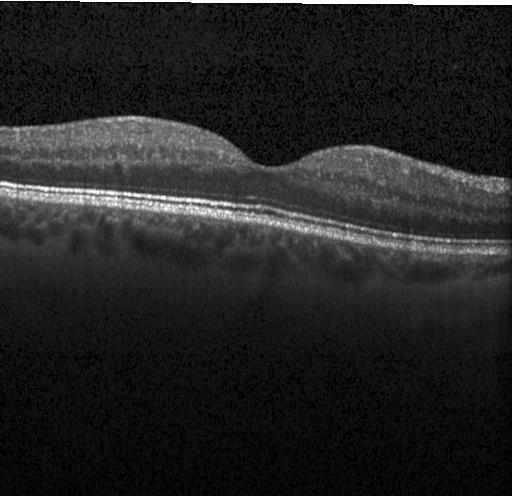 Finding: no choroidal neovascularization, no diabetic macular edema, and no drusen.